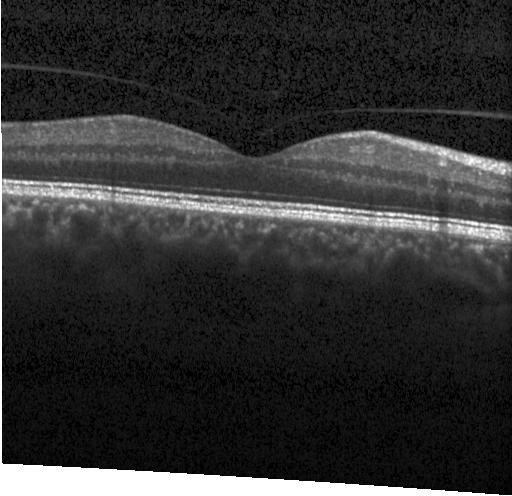 Spectral-domain OCT. Acquired on a Heidelberg Spectralis. Optical coherence tomography B-scan. Centered on the fovea
Neither choroidal neovascularization, diabetic macular edema, nor drusen.